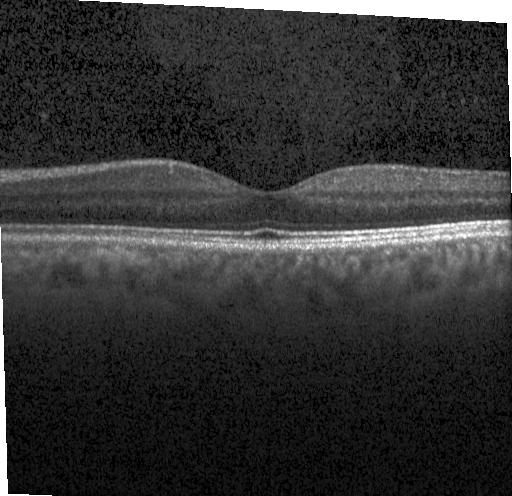
The scan shows no choroidal neovascularization, no diabetic macular edema, and no drusen.